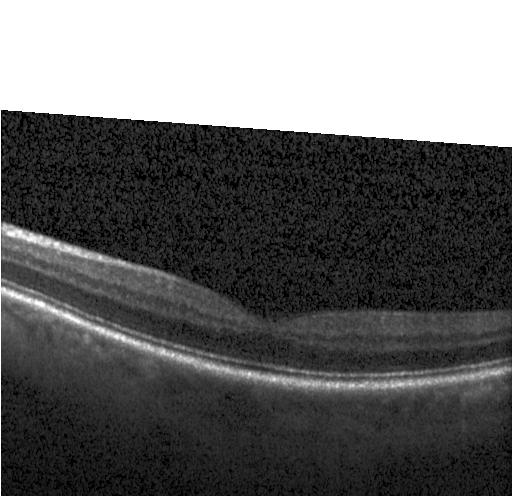

OCT line scan. Impression: neither choroidal neovascularization, diabetic macular edema, nor drusen.